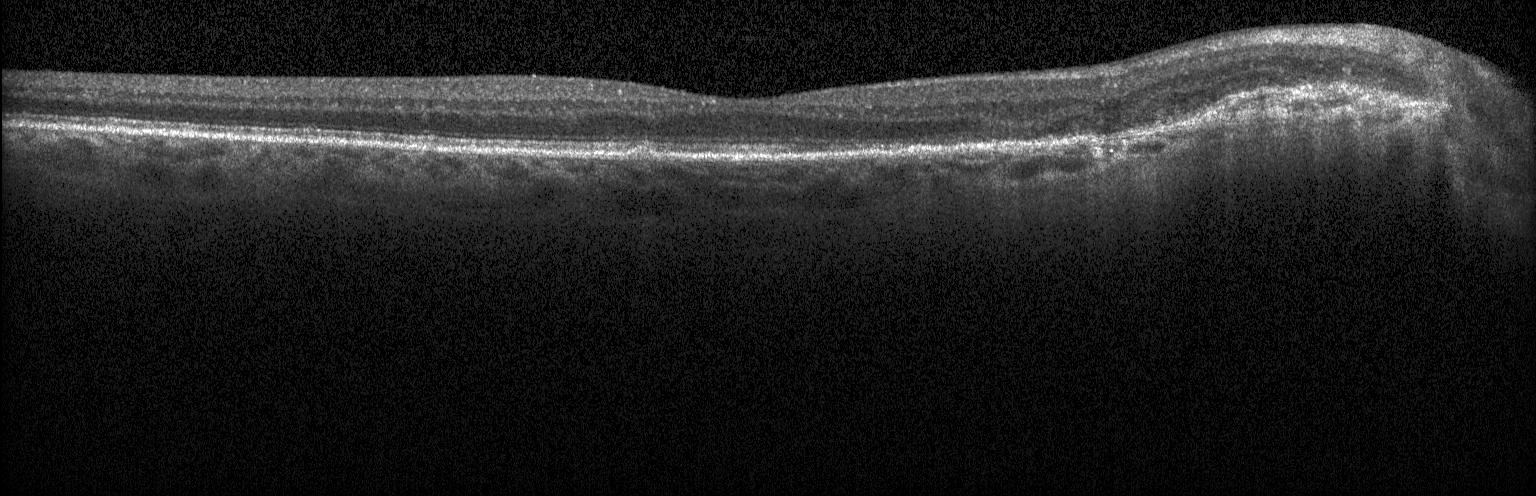 Retinal OCT cross-section.
Finding: a choroidal neovascular membrane.